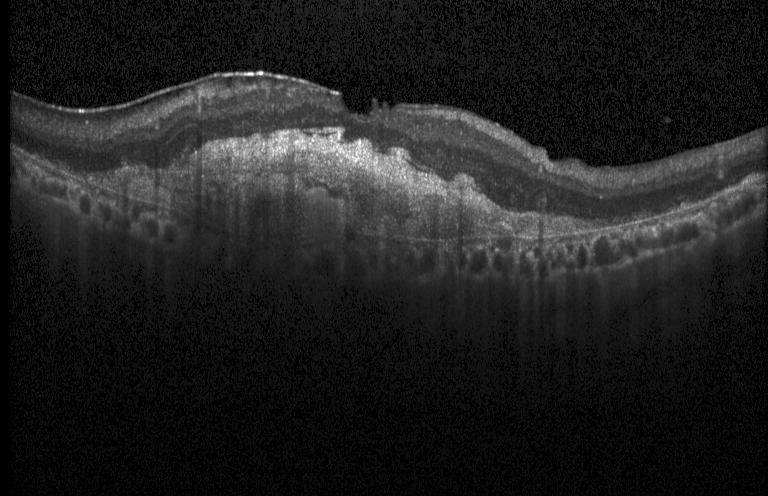
Dx: a choroidal neovascular membrane.